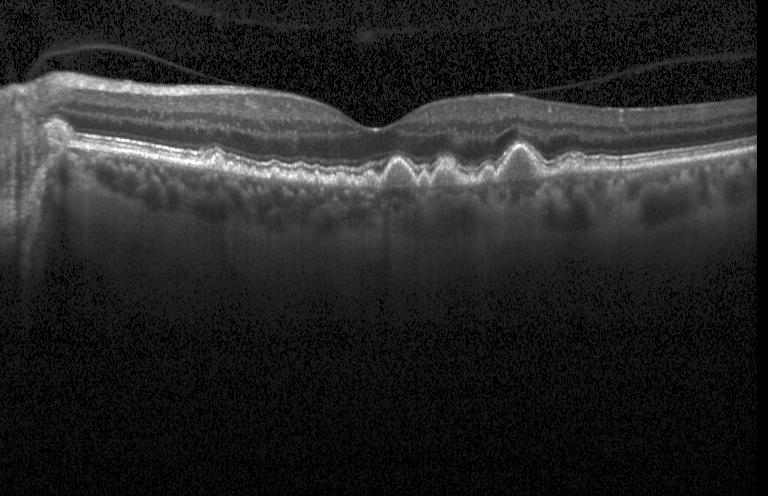 Acquired on a Heidelberg Spectralis; through the macula; retinal OCT B-scan.
OCT finding: sub-RPE drusenoid deposits.